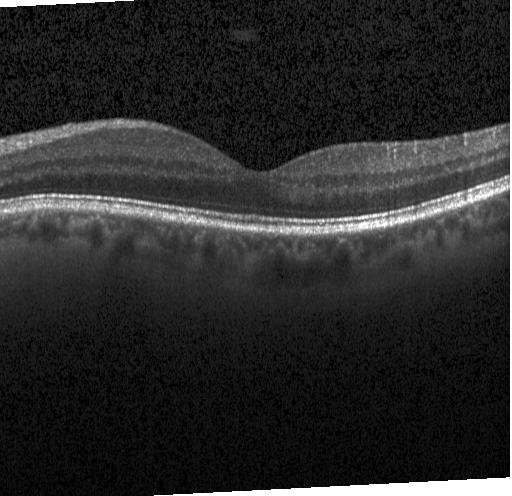

Finding: no choroidal neovascularization, diabetic macular edema, or drusen.